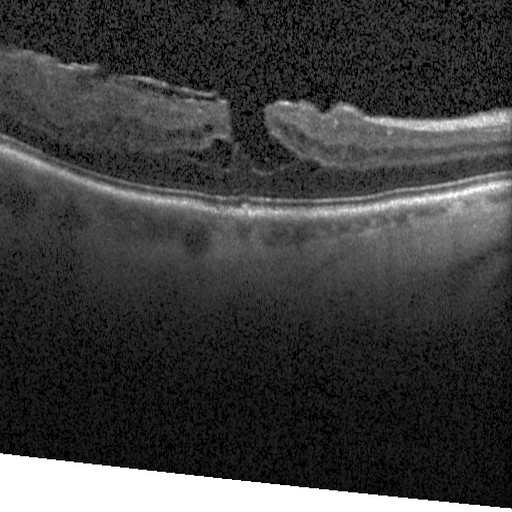 OCT B-scan, Heidelberg Spectralis OCT system — Impression: diabetic macular edema.